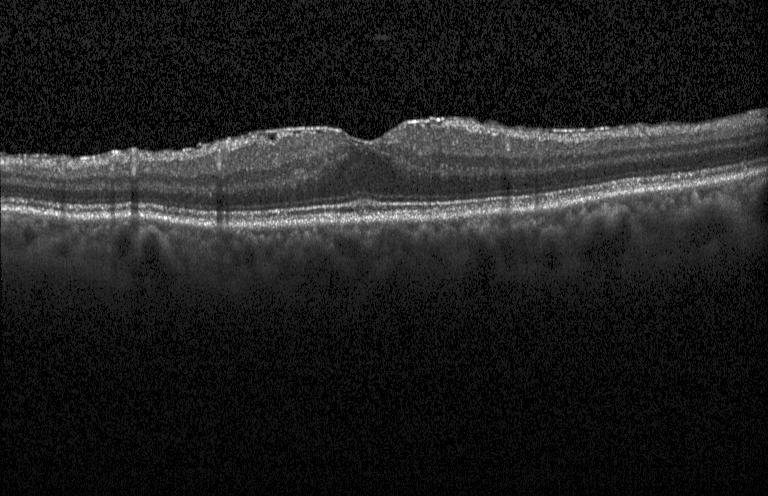

Dx: no choroidal neovascularization, diabetic macular edema, or drusen.